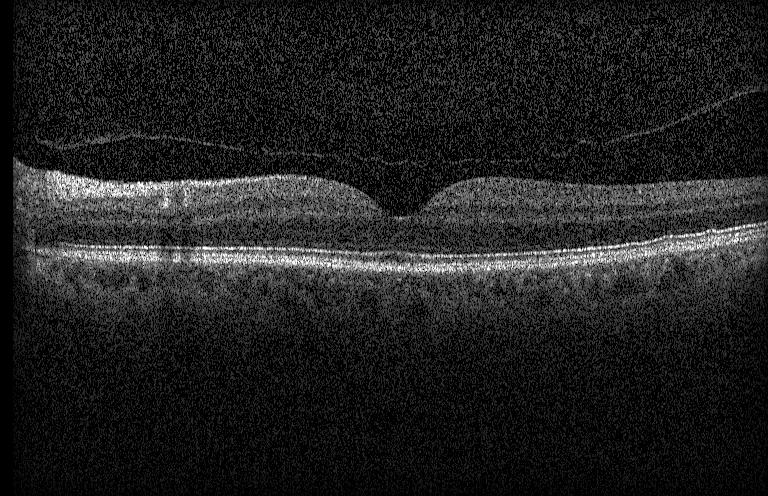 Retinal OCT B-scan
No evidence of CNV, DME, or drusen.